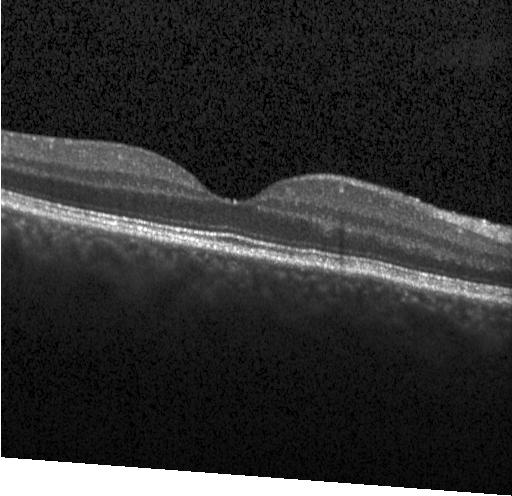 Macular scan. Spectral-domain OCT. Retinal OCT cross-section. Acquired on a Heidelberg Spectralis
Diagnosis: no evidence of CNV, DME, or drusen.